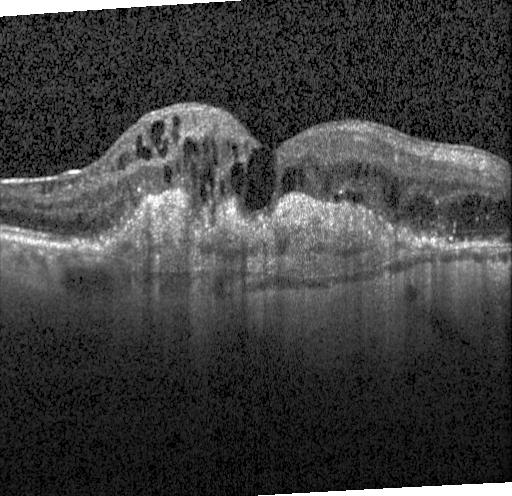

Impression: CNV.